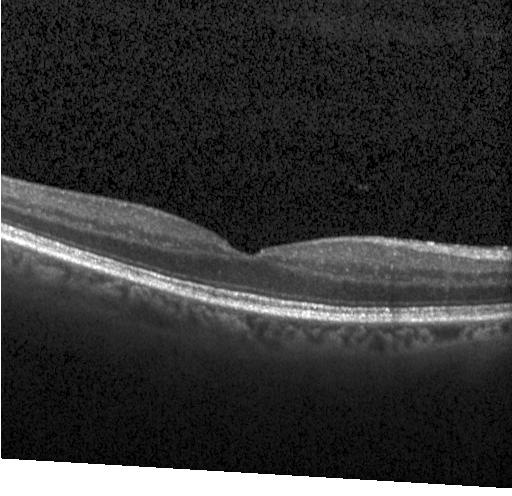 Diagnosis: neither choroidal neovascularization, diabetic macular edema, nor drusen.